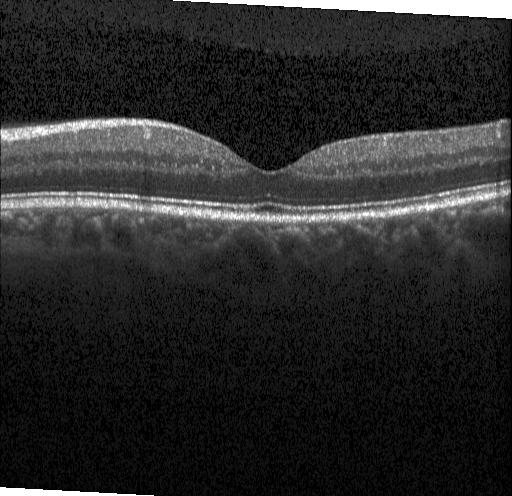 Retinal OCT B-scan; SD-OCT; horizontal scan through the fovea; acquired on a Heidelberg Spectralis.
Assessment: neither choroidal neovascularization, diabetic macular edema, nor drusen.